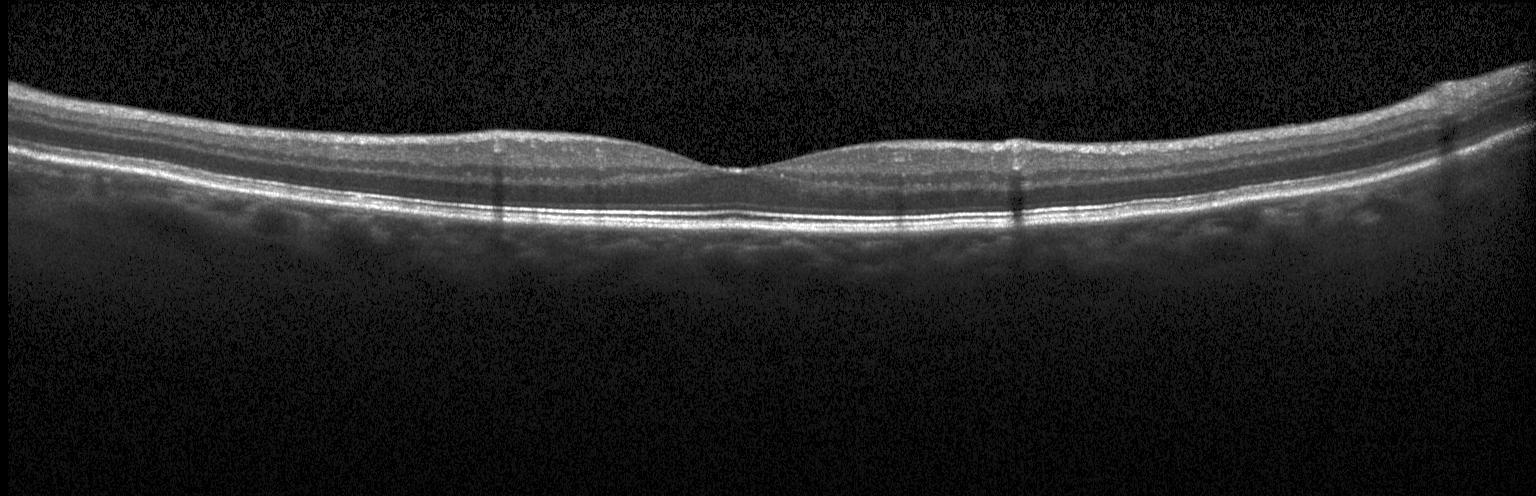
Optical coherence tomography B-scan, through the macula, SD-OCT, Heidelberg Spectralis OCT system.
Assessment: no choroidal neovascularization, no diabetic macular edema, and no drusen.